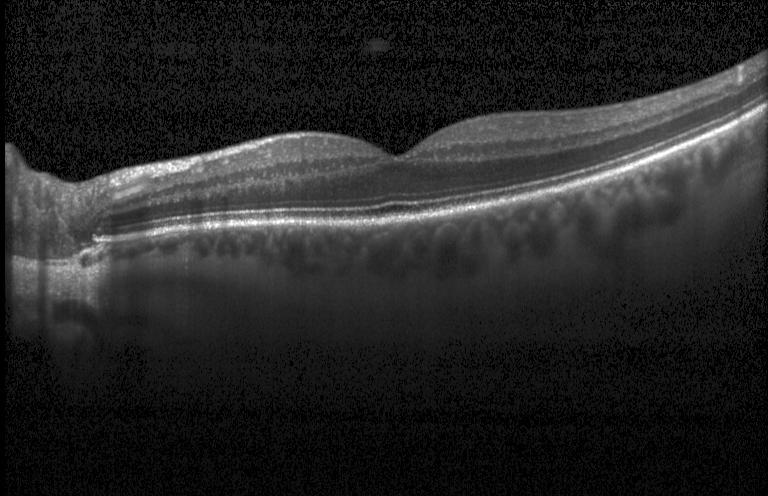

Optical coherence tomography scan.
Assessment: neither choroidal neovascularization, diabetic macular edema, nor drusen.